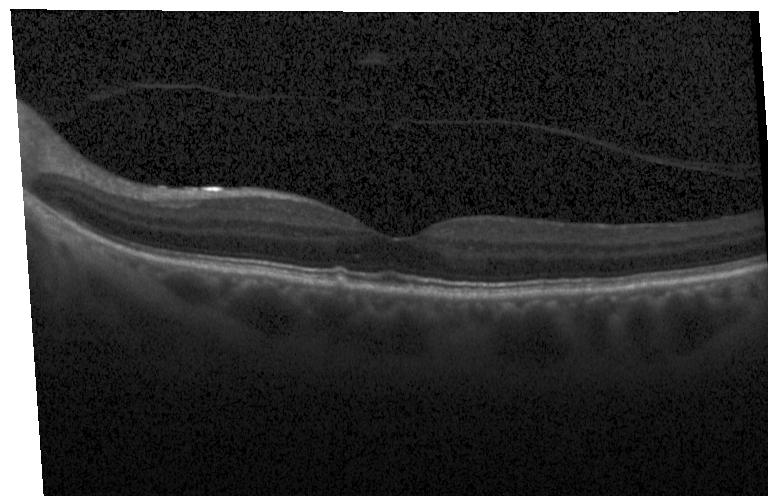 OCT finding: drusen.